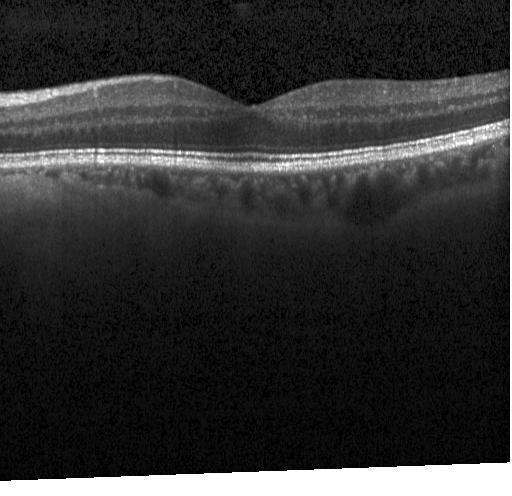

Finding: no choroidal neovascularization, diabetic macular edema, or drusen.